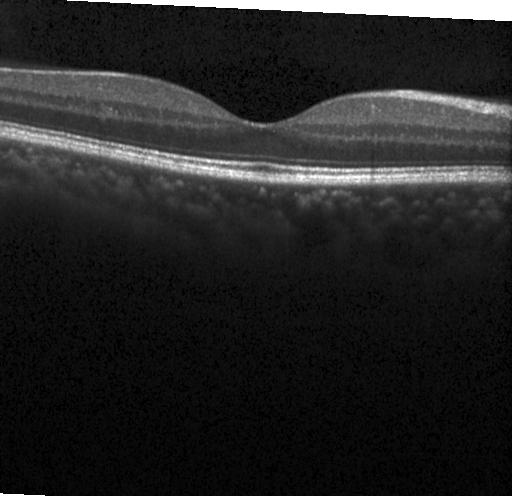
Instrument: Heidelberg Spectralis; optical coherence tomography scan.
Diagnosis: no choroidal neovascularization, diabetic macular edema, or drusen.